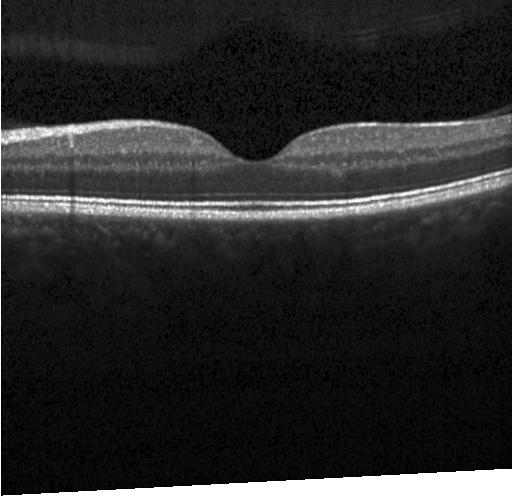
Impression: no choroidal neovascularization, diabetic macular edema, or drusen.